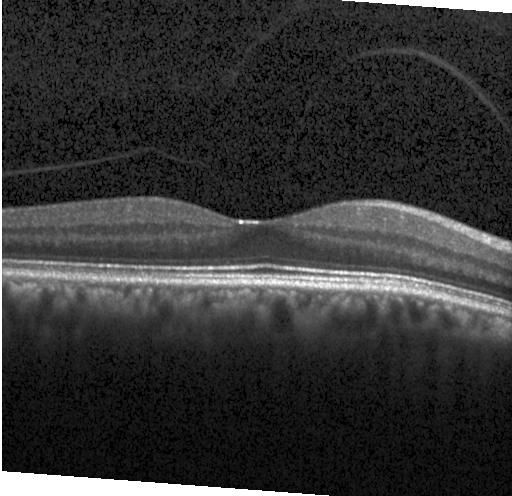
Finding: neither CNV, DME, nor drusen.